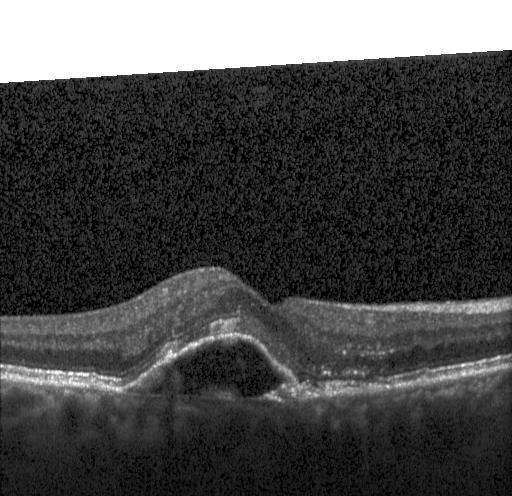

Impression: choroidal neovascularization.